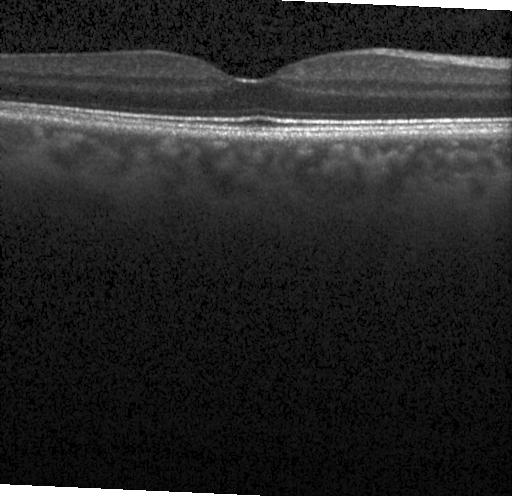

Optical coherence tomography B-scan · horizontal scan through the fovea · acquired on a Heidelberg Spectralis · spectral-domain optical coherence tomography — Diagnosis: neither CNV, DME, nor drusen.